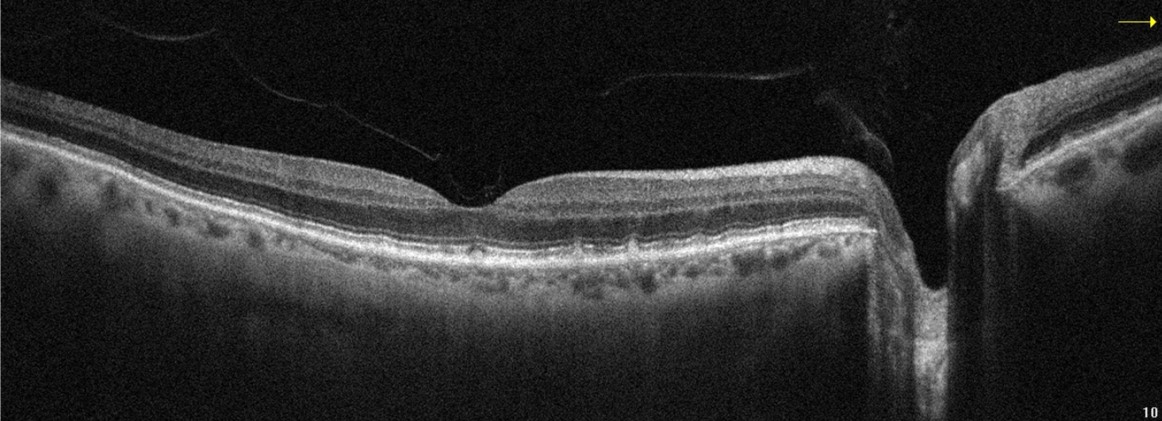 Macular OCT demonstrating age-related macular degeneration (AMD).